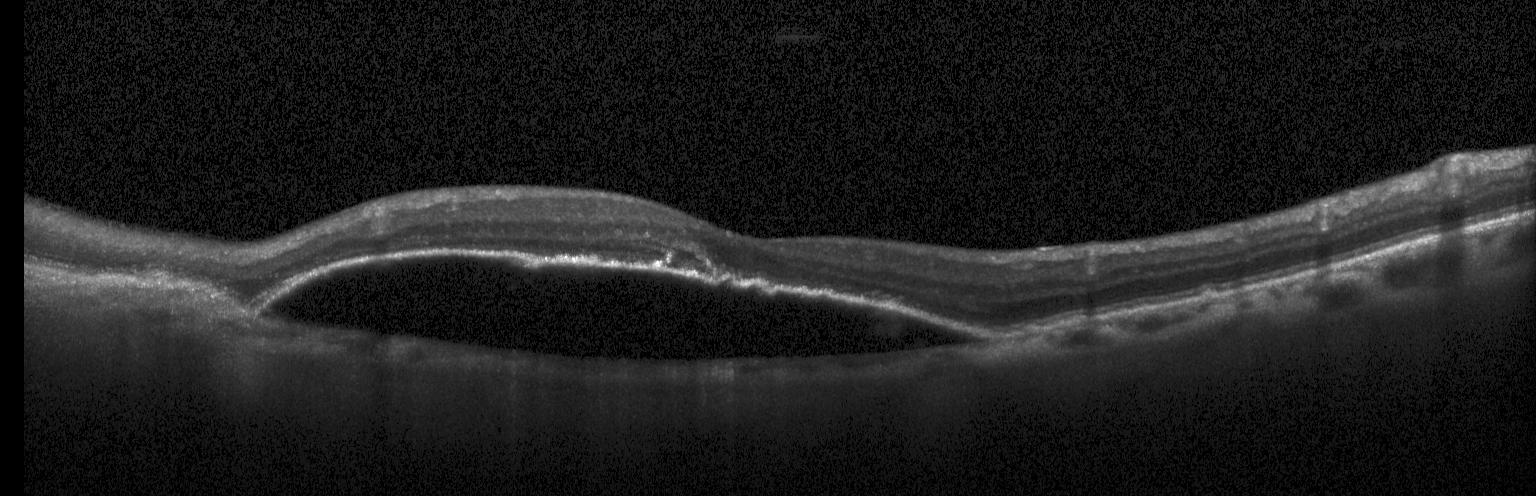
Optical coherence tomography scan, Heidelberg Spectralis, through the macula.
Diagnosis: a choroidal neovascular membrane.